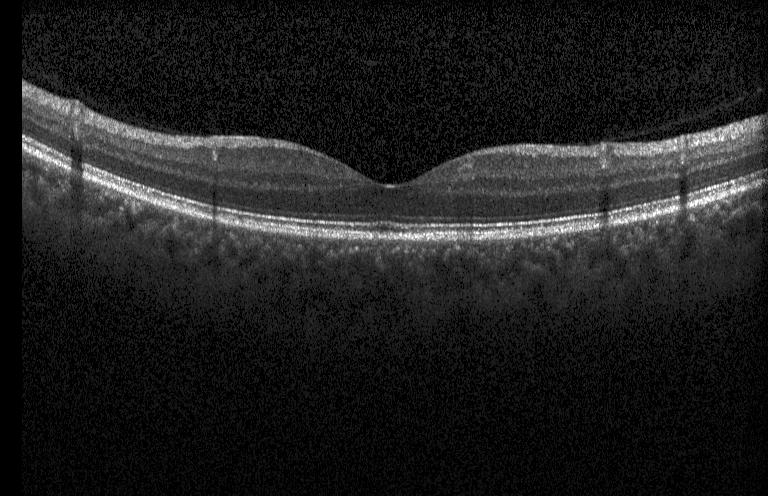
The scan shows no choroidal neovascularization, diabetic macular edema, or drusen.